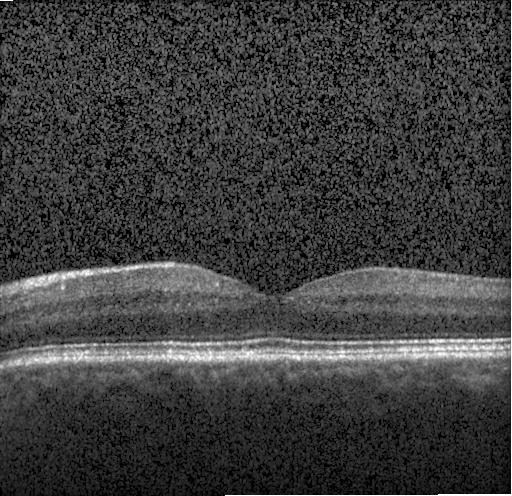 Impression: no choroidal neovascularization, no diabetic macular edema, and no drusen.